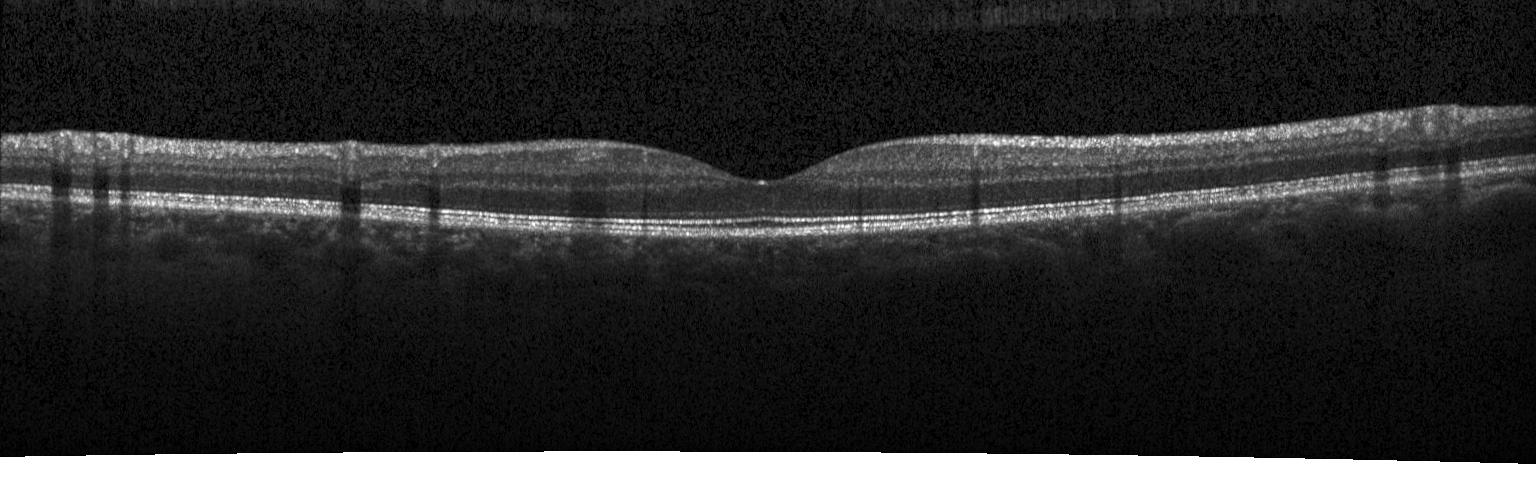

Spectral-domain OCT. Optical coherence tomography scan.
Dx: no choroidal neovascularization, diabetic macular edema, or drusen.